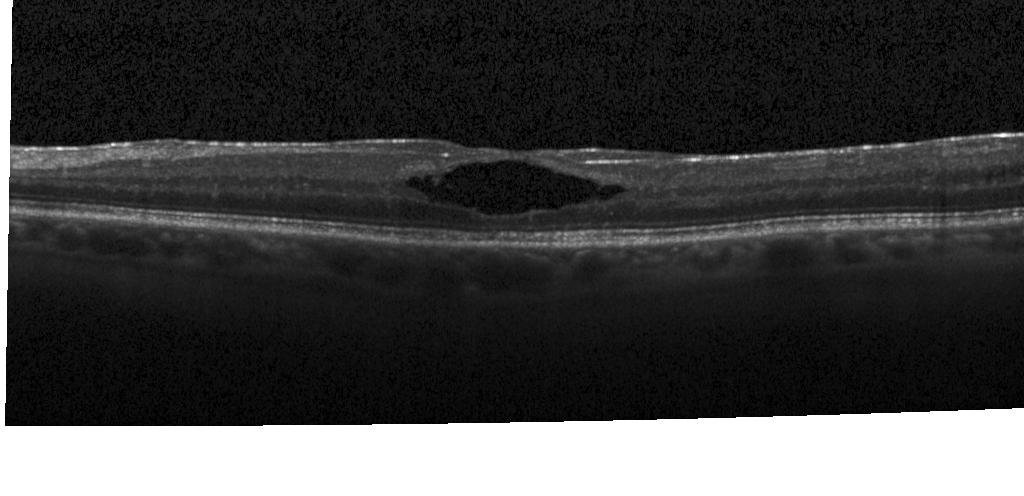 Retinal OCT cross-section, spectral-domain OCT. Impression: diabetic macular edema (DME).